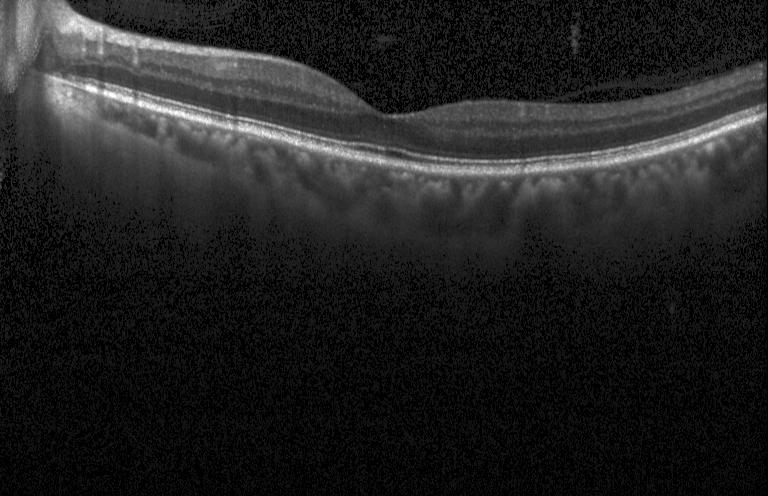
Horizontal scan through the fovea; spectral-domain optical coherence tomography; optical coherence tomography B-scan.
Diagnosis: no evidence of CNV, DME, or drusen.